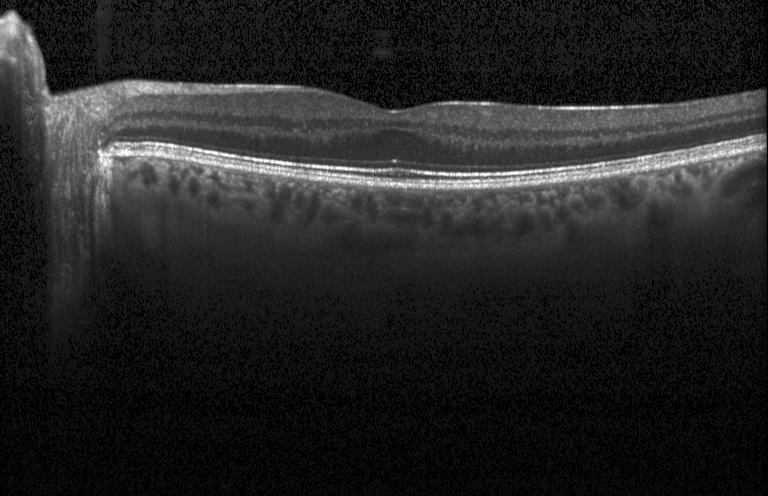

Acquired on a Heidelberg Spectralis · retinal OCT B-scan. Dx: no CNV, no DME, and no drusen.